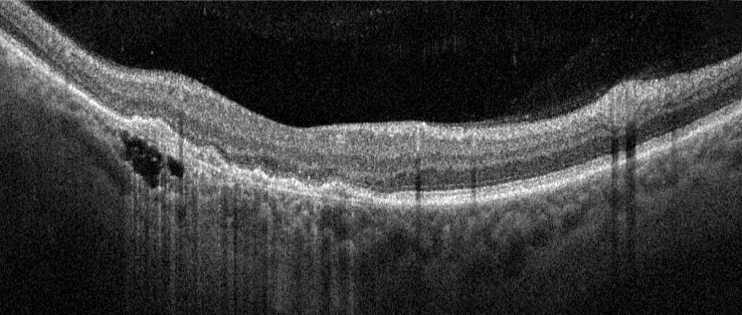 Assessment: age-related macular degeneration.